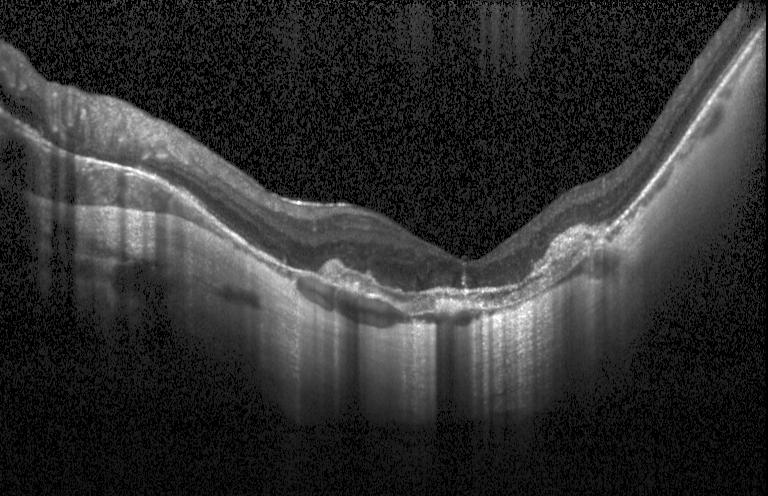

Optical coherence tomography scan. Impression: CNV.